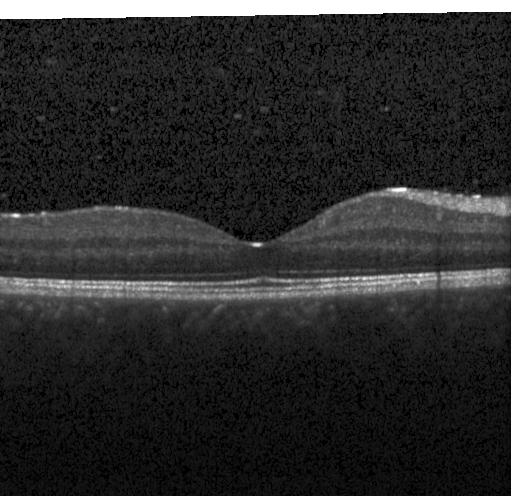
Macular OCT: no choroidal neovascularization, diabetic macular edema, or drusen.